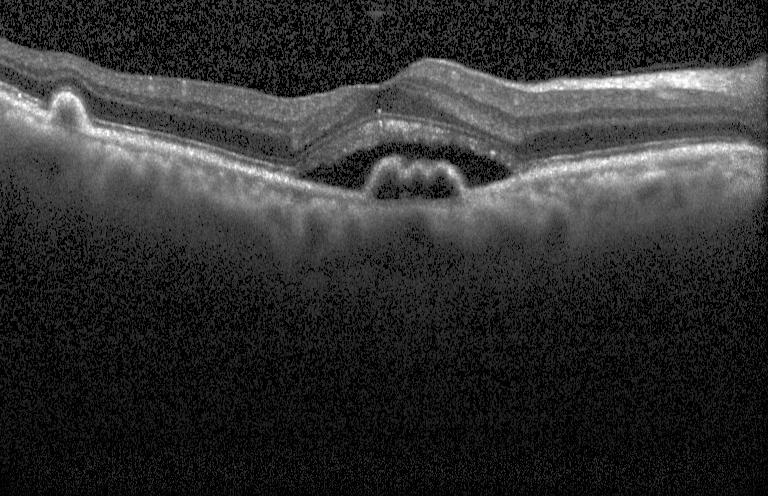

Finding: a choroidal neovascular membrane.